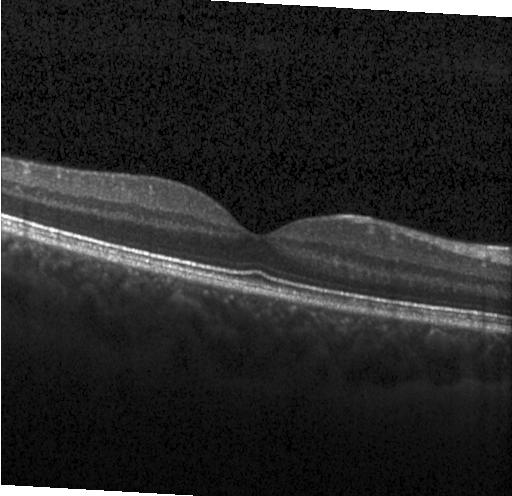

Retinal OCT cross-section showing no choroidal neovascularization, no diabetic macular edema, and no drusen.